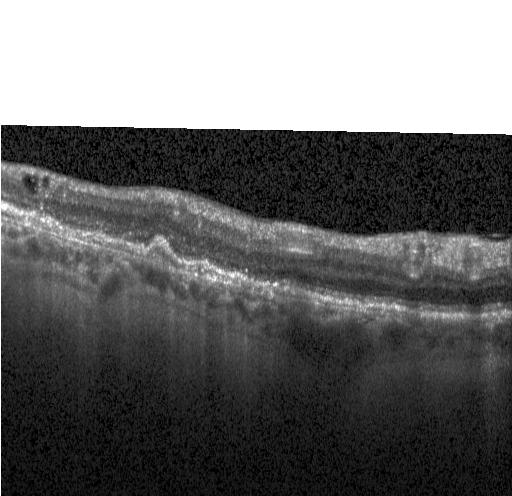

OCT line scan · spectral-domain optical coherence tomography — Finding: a choroidal neovascular membrane.